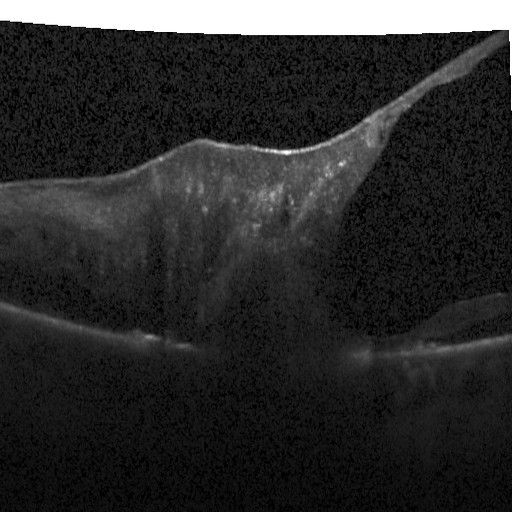
The scan shows diabetic macular edema.